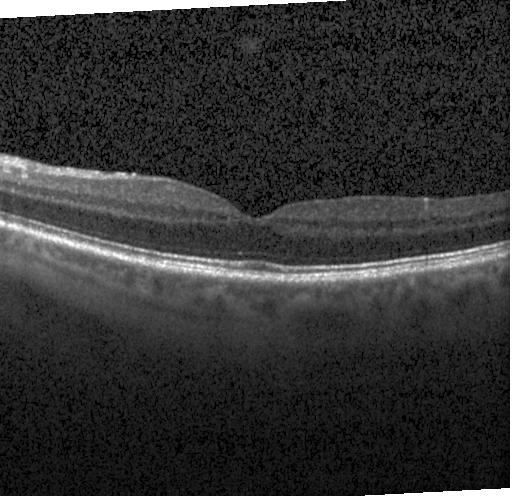
SD-OCT, through the macula, OCT line scan. Diagnosis: no choroidal neovascularization, no diabetic macular edema, and no drusen.